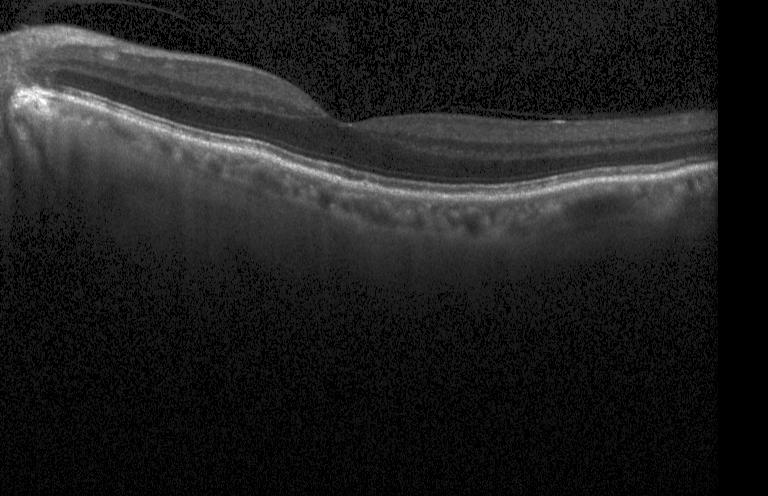 Spectral-domain OCT, OCT line scan, Heidelberg Spectralis OCT system. Impression: no choroidal neovascularization, no diabetic macular edema, and no drusen.